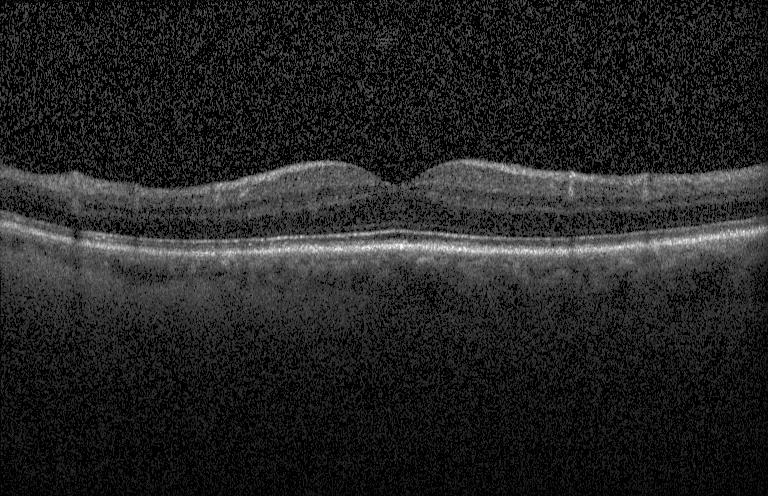 SD-OCT. Centered on the fovea. Heidelberg Spectralis OCT system. OCT line scan.
No CNV, DME, or drusen.